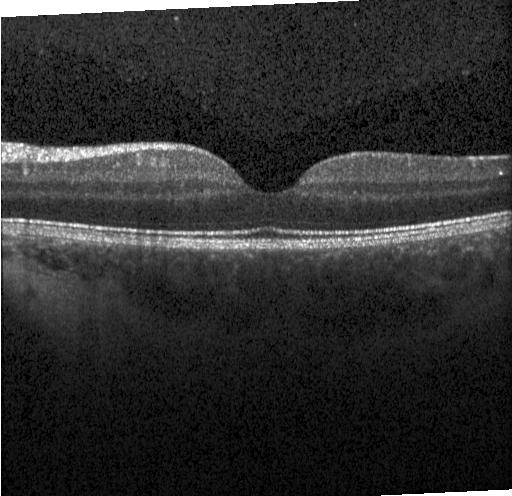 Retinal OCT cross-section · spectral-domain optical coherence tomography · instrument: Heidelberg Spectralis
Impression: no CNV, DME, or drusen.